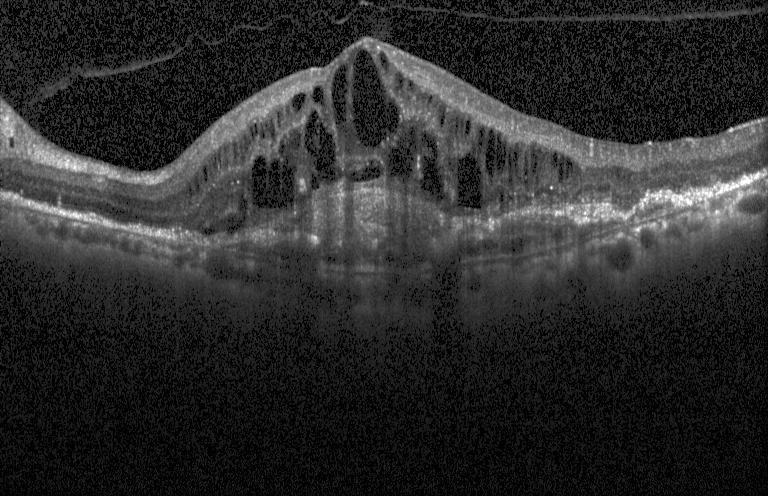 Heidelberg Spectralis, centered on the fovea, retinal OCT cross-section, spectral-domain OCT. Impression: choroidal neovascularization.